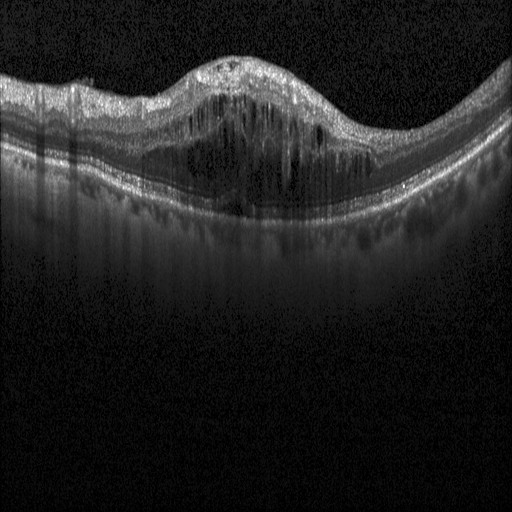

OCT line scan — The scan shows diabetic macular edema (DME).